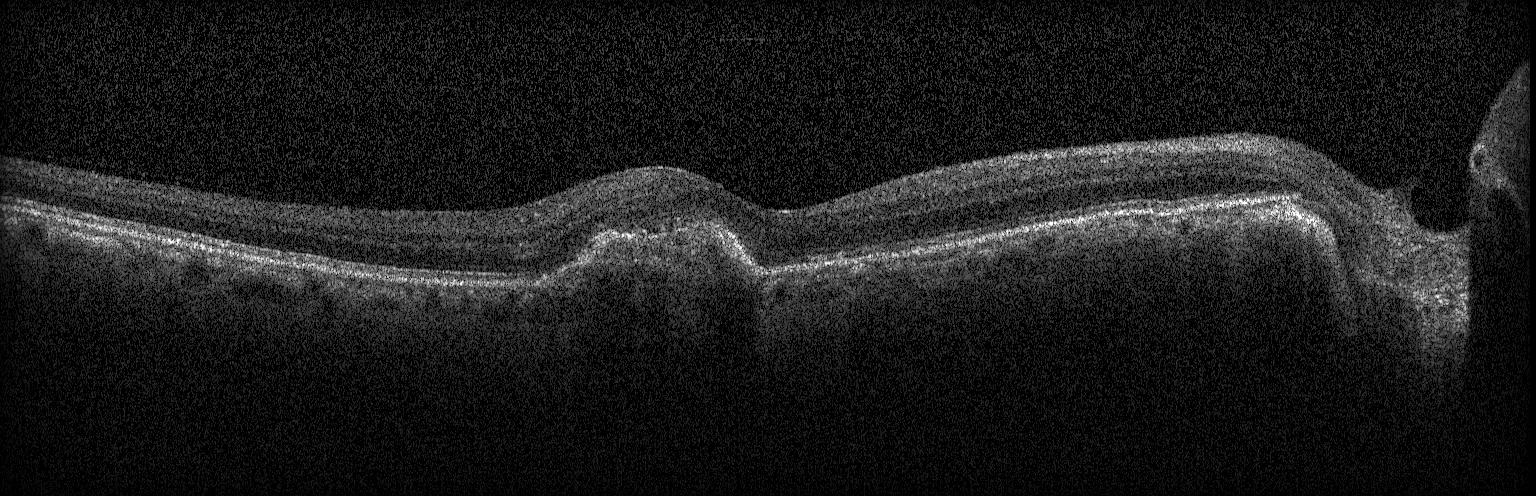
Retinal OCT cross-section. SD-OCT — Dx: CNV.